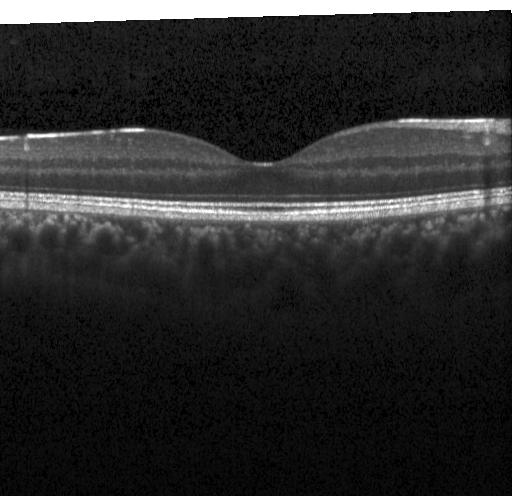

Spectral-domain OCT; Heidelberg Spectralis; OCT B-scan.
This B-scan demonstrates no CNV, no DME, and no drusen.